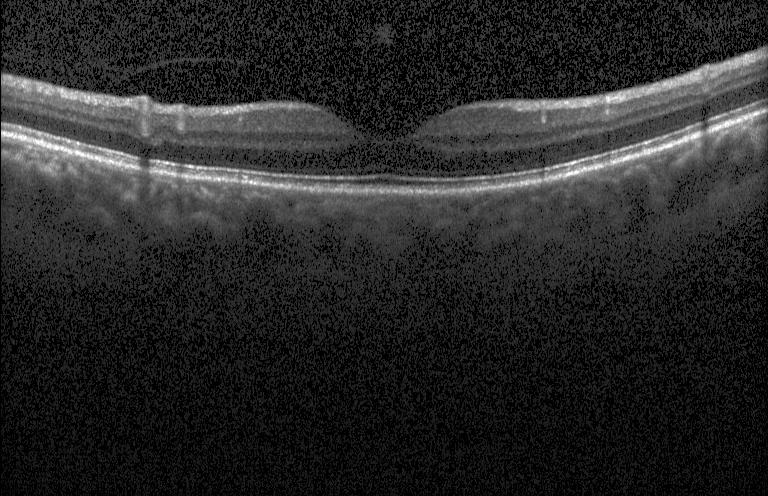 Macular OCT: neither choroidal neovascularization, diabetic macular edema, nor drusen.